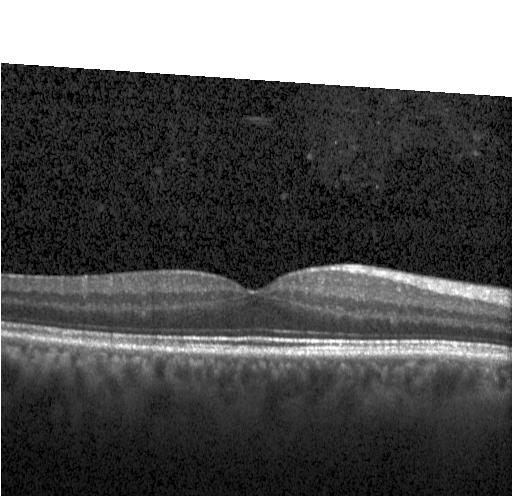 Optical coherence tomography B-scan · SD-OCT · macular scan · acquired on a Heidelberg Spectralis. Finding: neither choroidal neovascularization, diabetic macular edema, nor drusen.